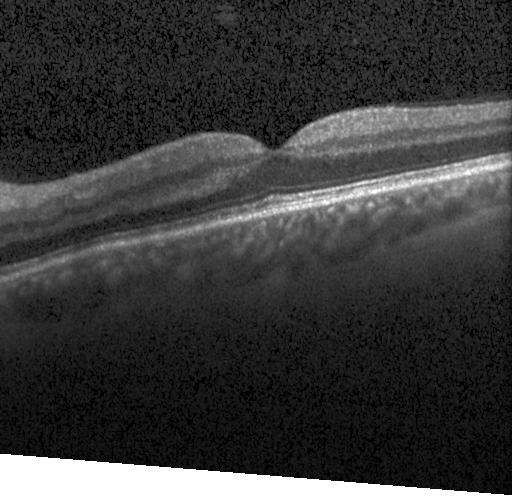

OCT B-scan. Through the macula. Spectral-domain optical coherence tomography. Instrument: Heidelberg Spectralis
Dx: no CNV, DME, or drusen.